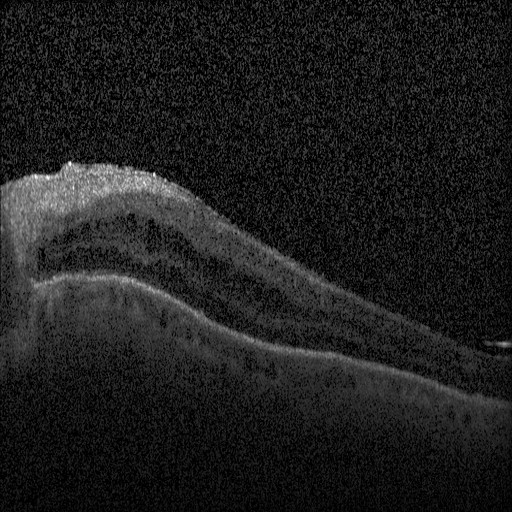

Heidelberg Spectralis, OCT line scan, macular scan. Assessment: diabetic macular edema (DME).